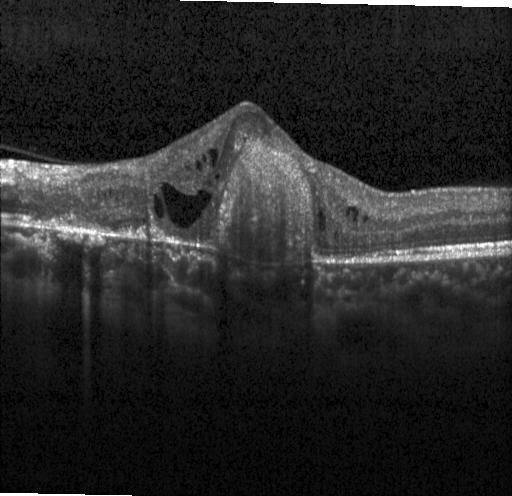

Fovea-centered; retinal OCT B-scan; Heidelberg Spectralis; spectral-domain optical coherence tomography — Finding: a choroidal neovascular membrane.